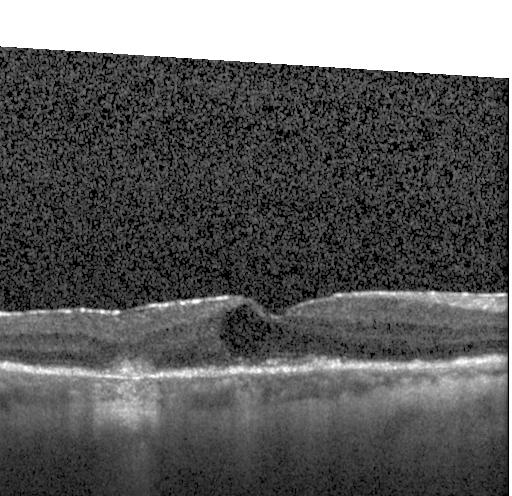

Fovea-centered. Spectral-domain optical coherence tomography. OCT B-scan. Heidelberg Spectralis OCT system. Assessment: a choroidal neovascular membrane.